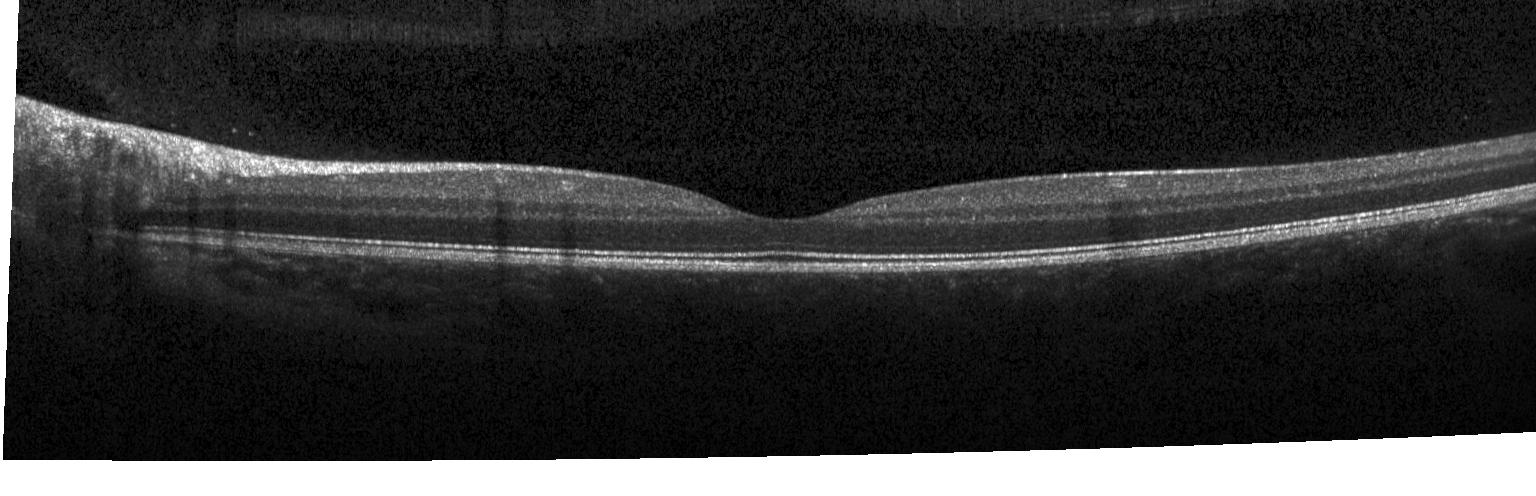

Spectral-domain optical coherence tomography · Heidelberg Spectralis · OCT B-scan. Impression: no CNV, DME, or drusen.